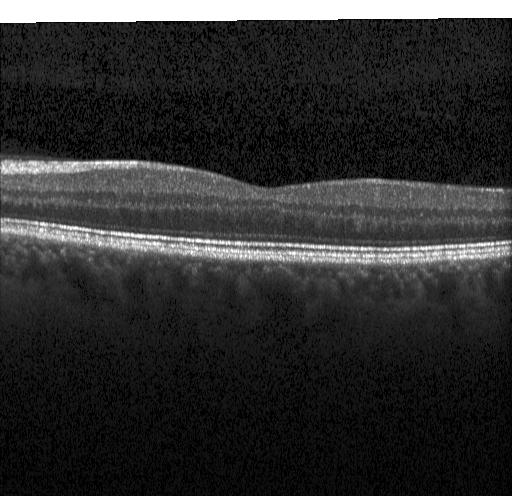

Through the macula · acquired on a Heidelberg Spectralis · SD-OCT · retinal OCT B-scan. Impression: no choroidal neovascularization, no diabetic macular edema, and no drusen.